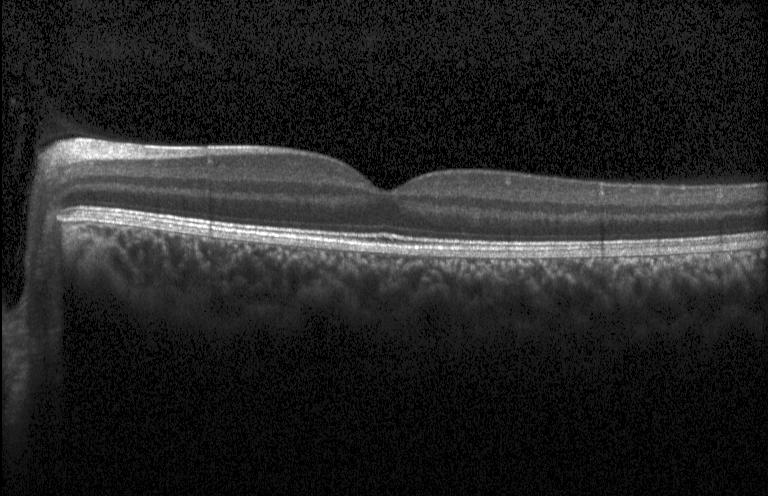 SD-OCT. OCT line scan. Acquired on a Heidelberg Spectralis. Horizontal scan through the fovea
Impression: no choroidal neovascularization, no diabetic macular edema, and no drusen.